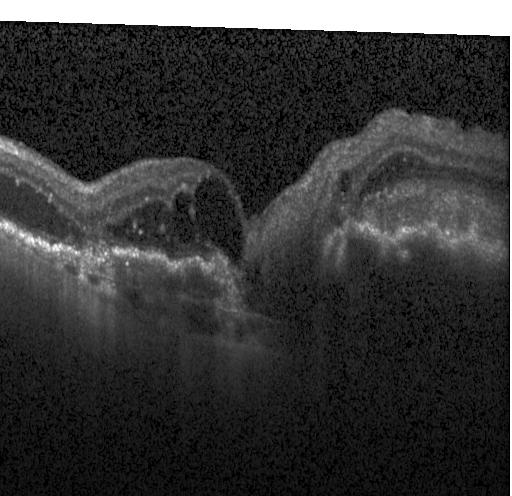
Retinal OCT B-scan, spectral-domain optical coherence tomography — CNV.